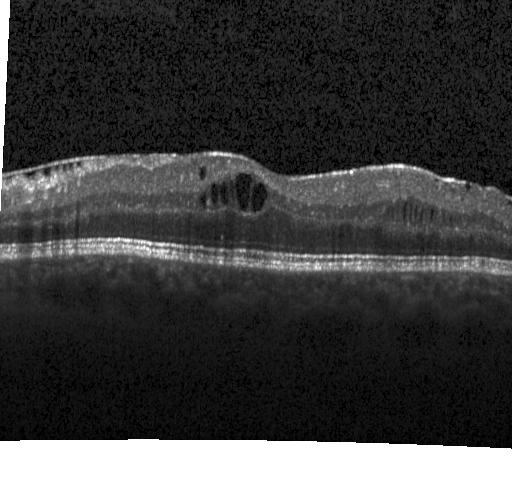

Retinal OCT B-scan — This B-scan demonstrates diabetic macular edema (DME).